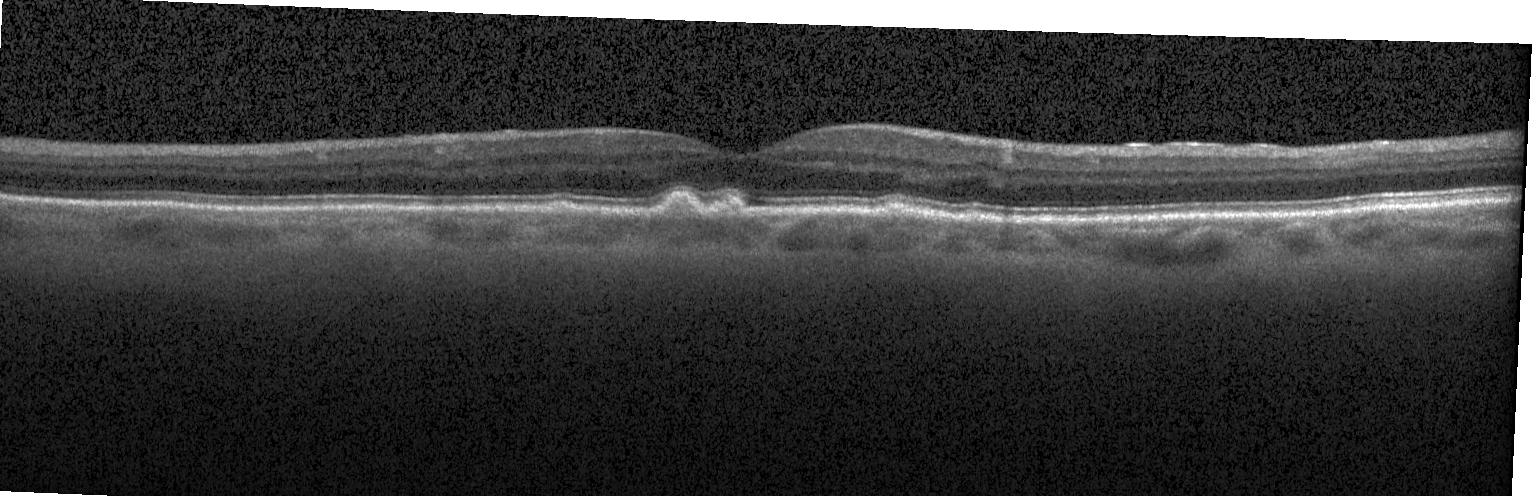

Centered on the fovea · spectral-domain optical coherence tomography · acquired on a Heidelberg Spectralis · optical coherence tomography B-scan — Sub-RPE drusenoid deposits.